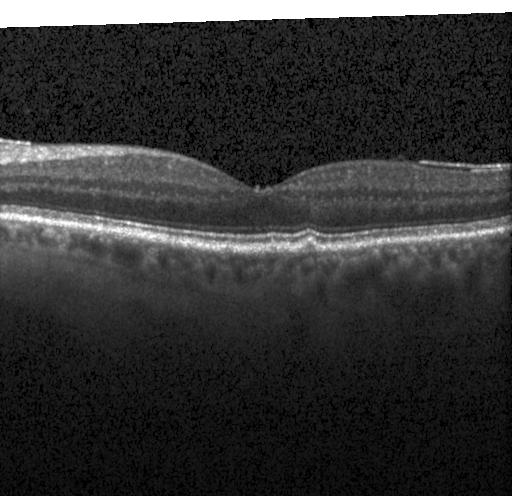

Spectral-domain optical coherence tomography, optical coherence tomography B-scan, through the macula, acquired on a Heidelberg Spectralis.
Macular OCT: drusen.